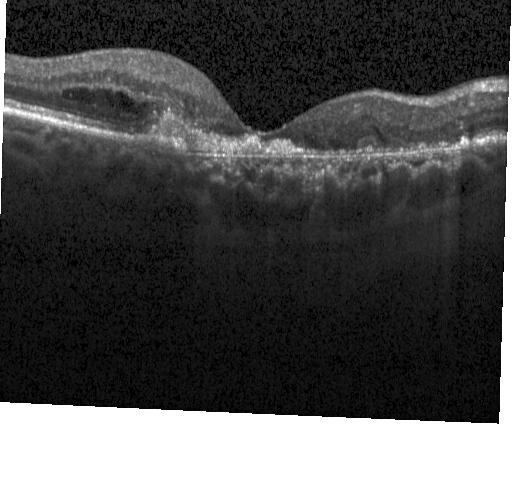
Macular scan; spectral-domain optical coherence tomography; retinal OCT B-scan; acquired on a Heidelberg Spectralis. Macular OCT: a choroidal neovascular membrane.